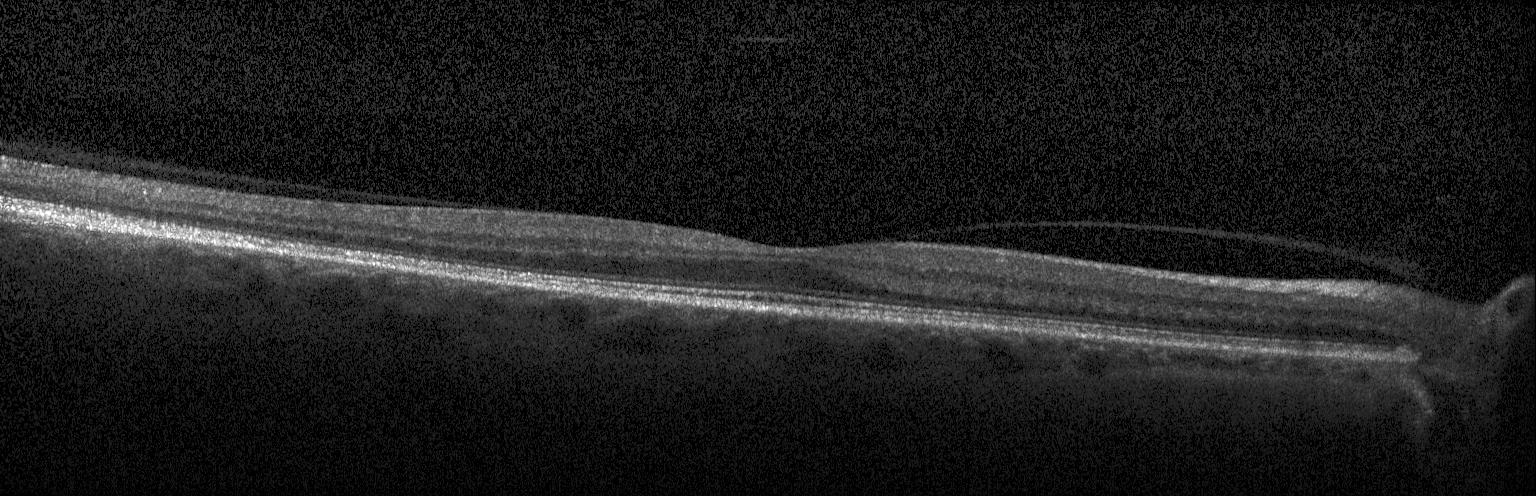
OCT B-scan showing no choroidal neovascularization, no diabetic macular edema, and no drusen.